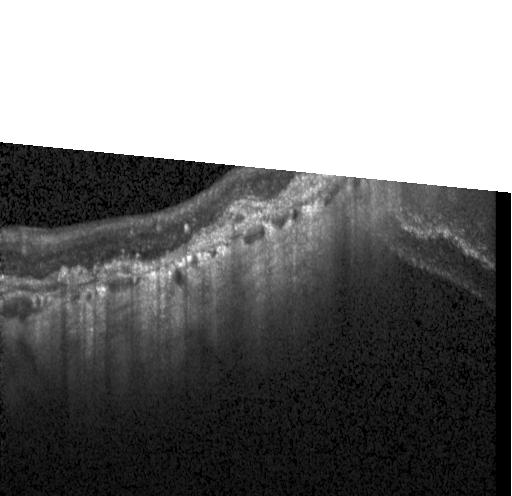 Dx: a choroidal neovascular membrane.